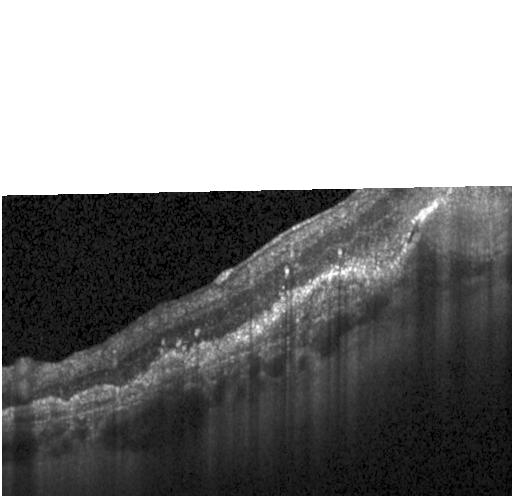

Instrument: Heidelberg Spectralis; optical coherence tomography B-scan
Macular OCT: a choroidal neovascular membrane.